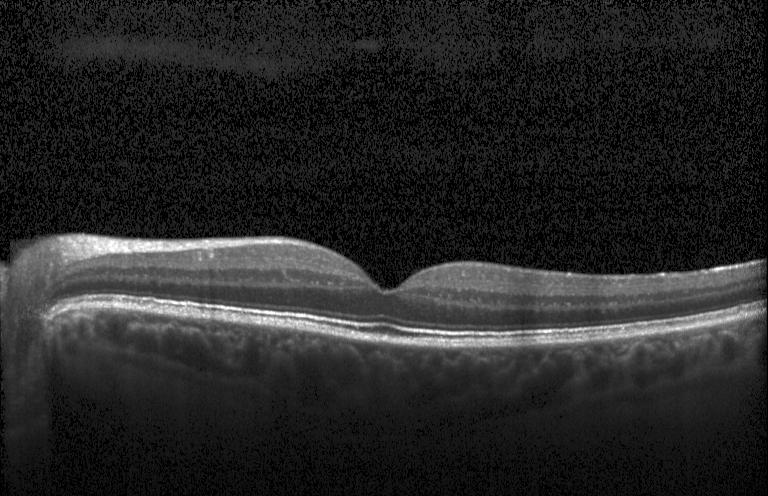
This B-scan demonstrates no choroidal neovascularization, diabetic macular edema, or drusen.